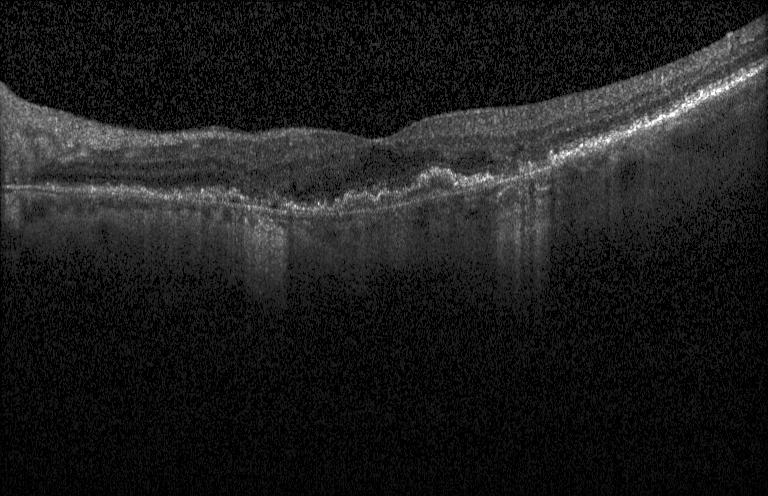
OCT line scan.
OCT finding: choroidal neovascularization.